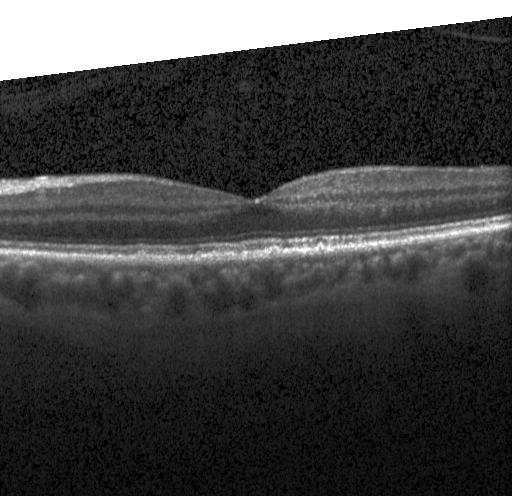 Sub-RPE drusenoid deposits.